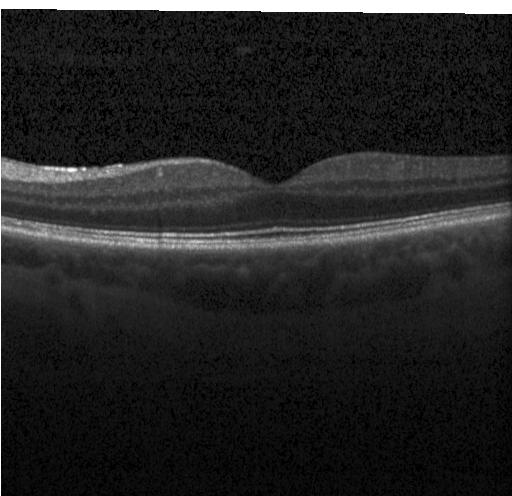
Optical coherence tomography B-scan · centered on the fovea · spectral-domain OCT · acquired on a Heidelberg Spectralis. Impression: neither choroidal neovascularization, diabetic macular edema, nor drusen.